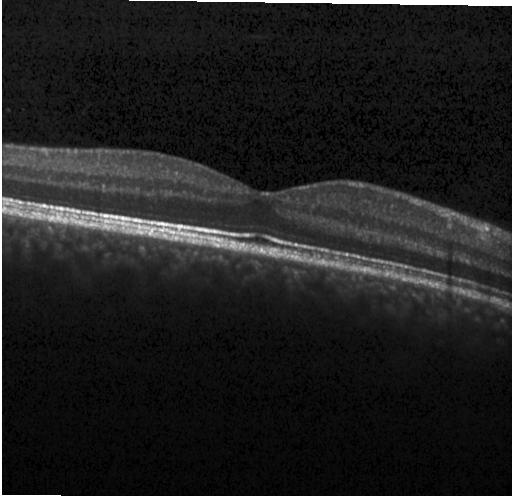
Through the macula, Heidelberg Spectralis, OCT line scan. OCT finding: no evidence of choroidal neovascularization, diabetic macular edema, or drusen.